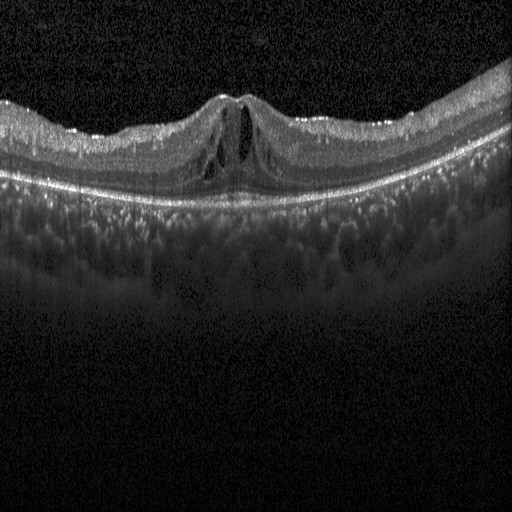 Optical coherence tomography scan, spectral-domain optical coherence tomography, centered on the fovea, acquired on a Heidelberg Spectralis — Dx: diabetic macular edema (DME).